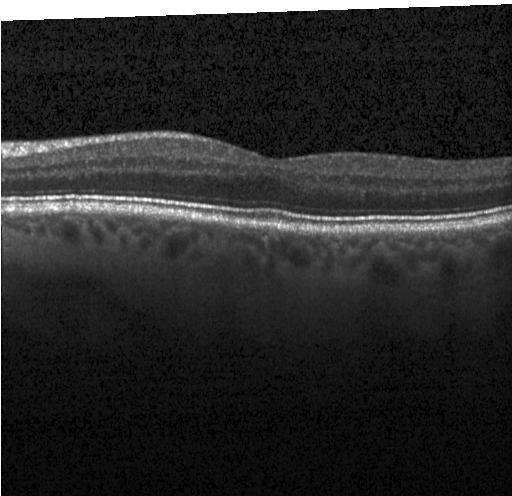

OCT finding: neither CNV, DME, nor drusen.